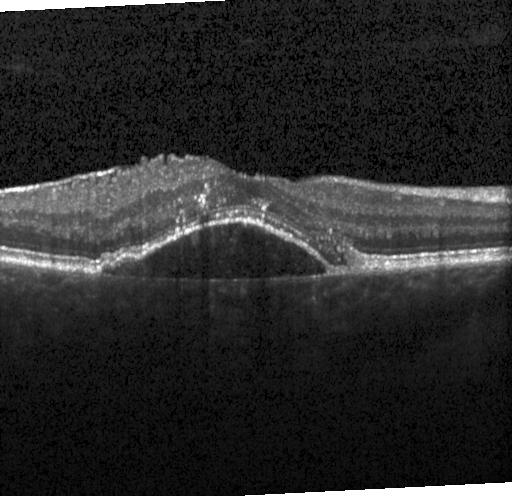

Instrument: Heidelberg Spectralis; optical coherence tomography scan; horizontal scan through the fovea — Assessment: CNV.